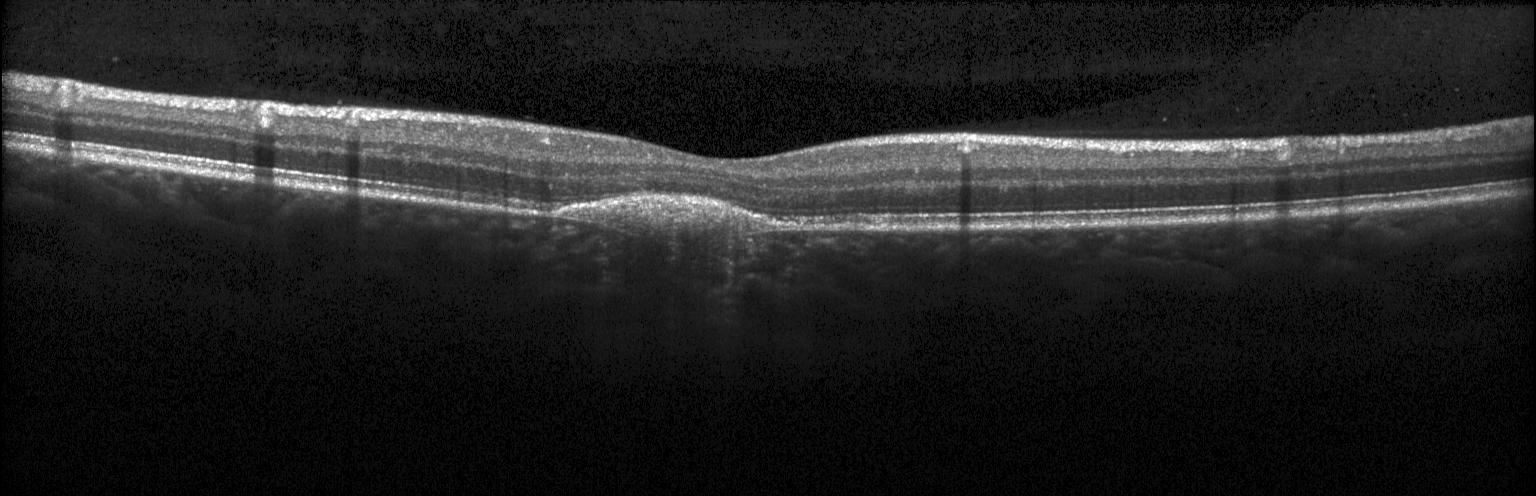 OCT B-scan showing choroidal neovascularization (CNV).